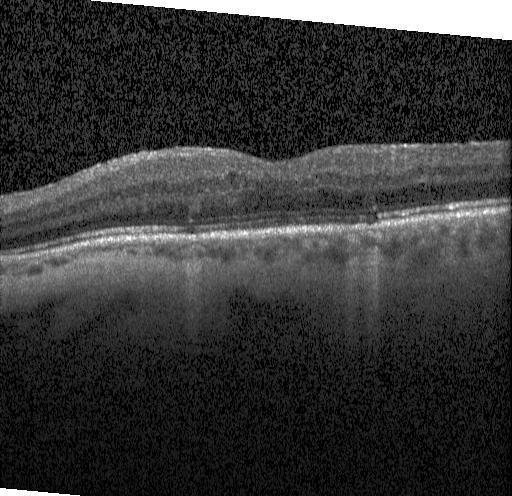
Retinal OCT B-scan; instrument: Heidelberg Spectralis.
Diagnosis: no CNV, DME, or drusen.